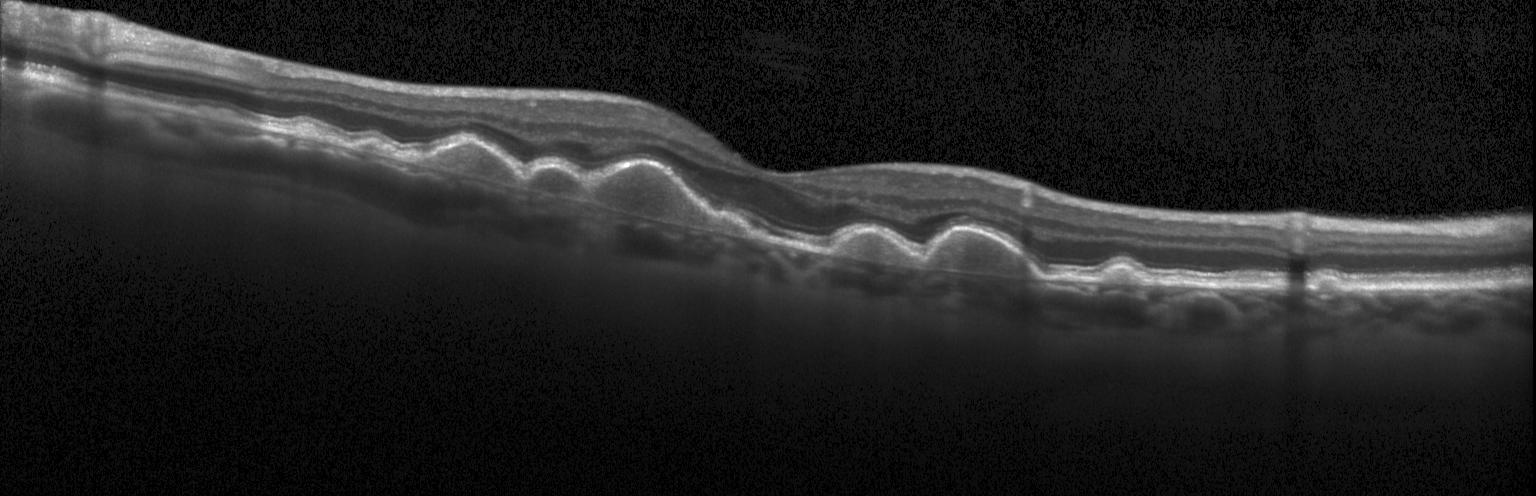

Sub-RPE drusenoid deposits.